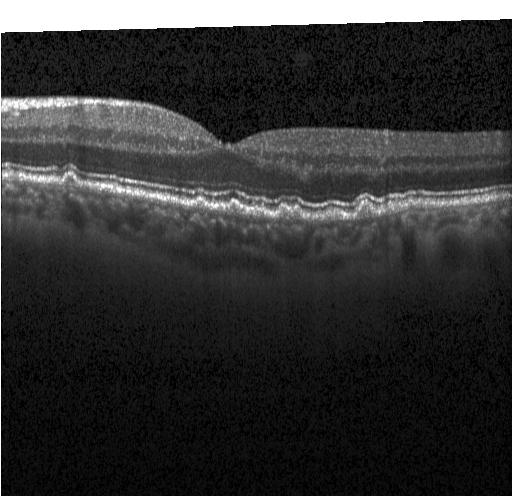

OCT line scan. Acquired on a Heidelberg Spectralis. SD-OCT — Finding: multiple drusen.